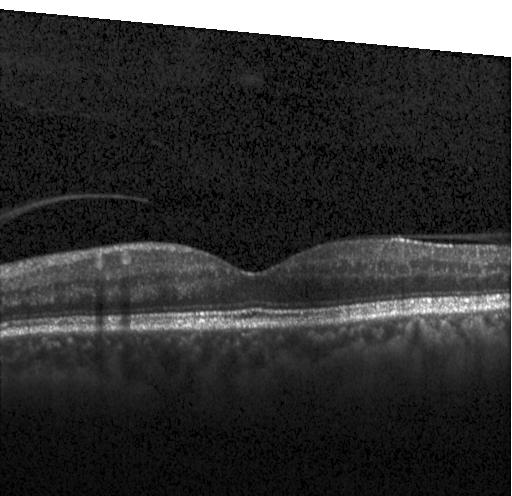 Heidelberg Spectralis OCT system; optical coherence tomography B-scan.
Diagnosis: no evidence of choroidal neovascularization, diabetic macular edema, or drusen.